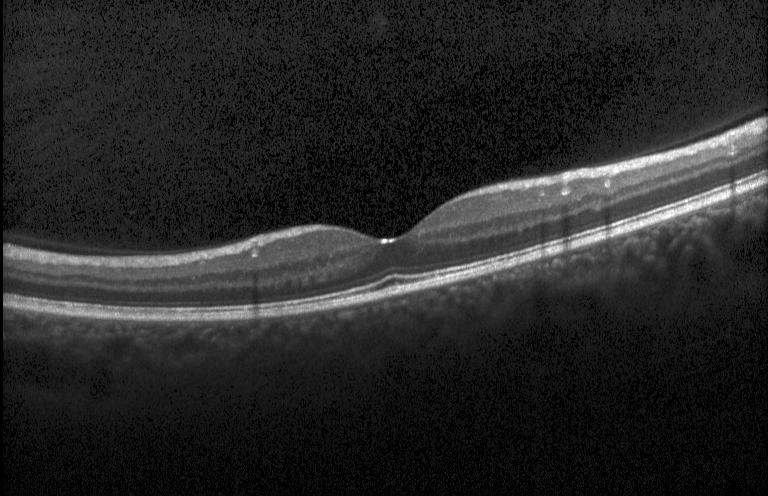

Retinal OCT B-scan — Finding: neither choroidal neovascularization, diabetic macular edema, nor drusen.